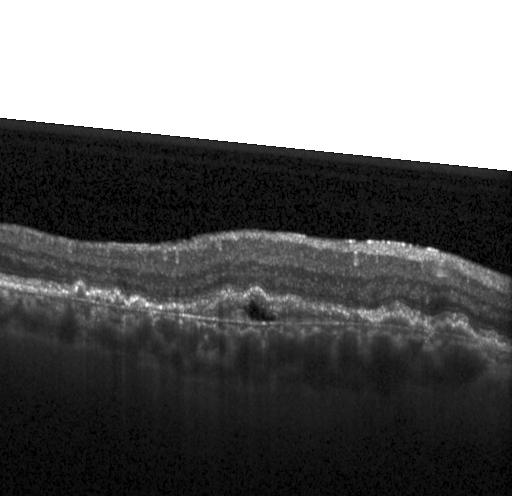
Spectral-domain optical coherence tomography, OCT B-scan, instrument: Heidelberg Spectralis. Diagnosis: choroidal neovascularization (CNV).